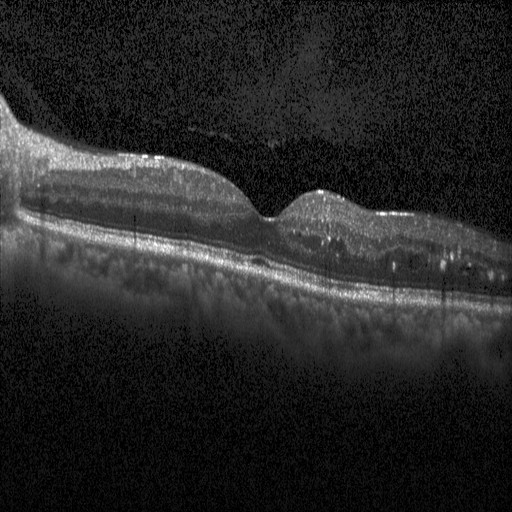
Horizontal scan through the fovea · instrument: Heidelberg Spectralis · OCT line scan · spectral-domain OCT
The scan shows diabetic macular edema (DME).